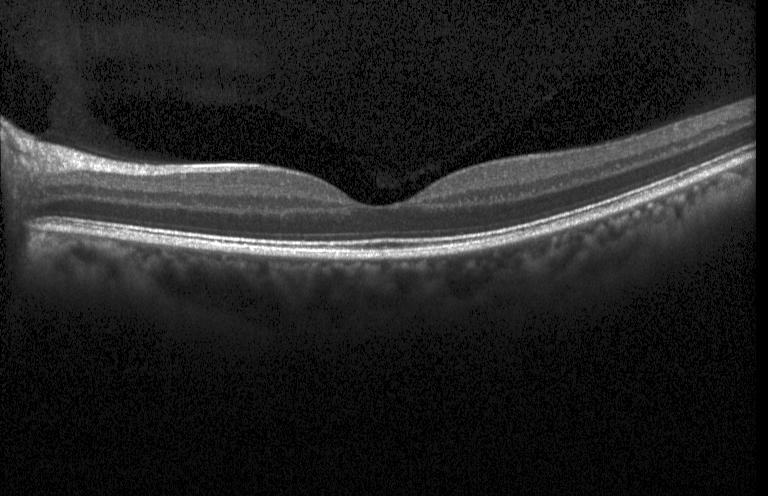
SD-OCT; optical coherence tomography B-scan; Heidelberg Spectralis OCT system; macular scan
Diagnosis: neither choroidal neovascularization, diabetic macular edema, nor drusen.